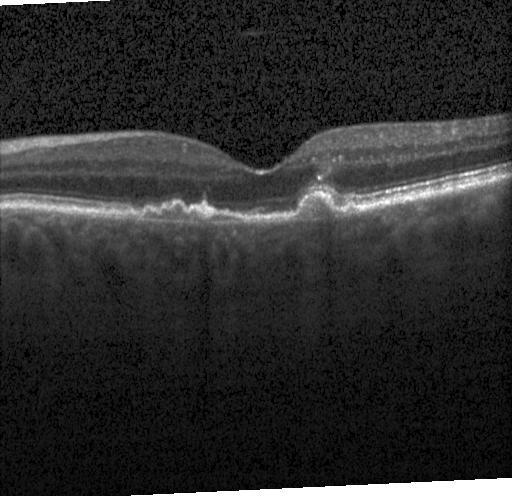
Finding: a choroidal neovascular membrane.